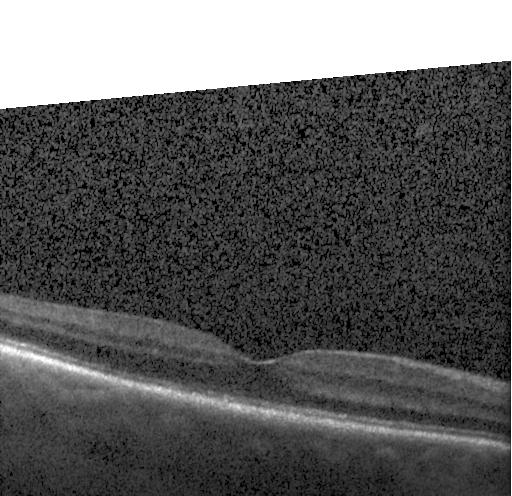

Diagnosis: no evidence of choroidal neovascularization, diabetic macular edema, or drusen.